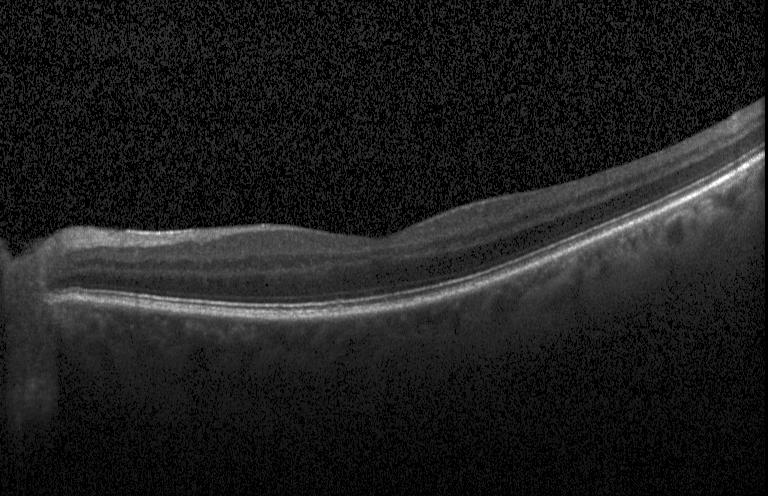

OCT B-scan, Heidelberg Spectralis OCT system, spectral-domain OCT — No CNV, DME, or drusen.